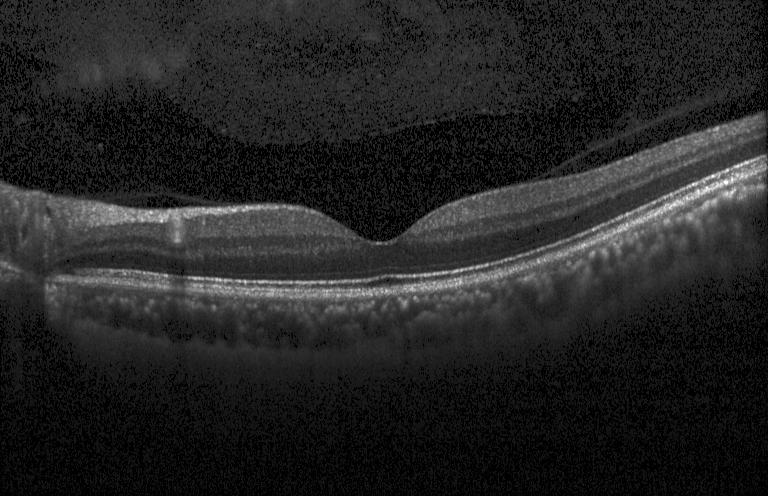

OCT line scan.
OCT finding: no choroidal neovascularization, no diabetic macular edema, and no drusen.